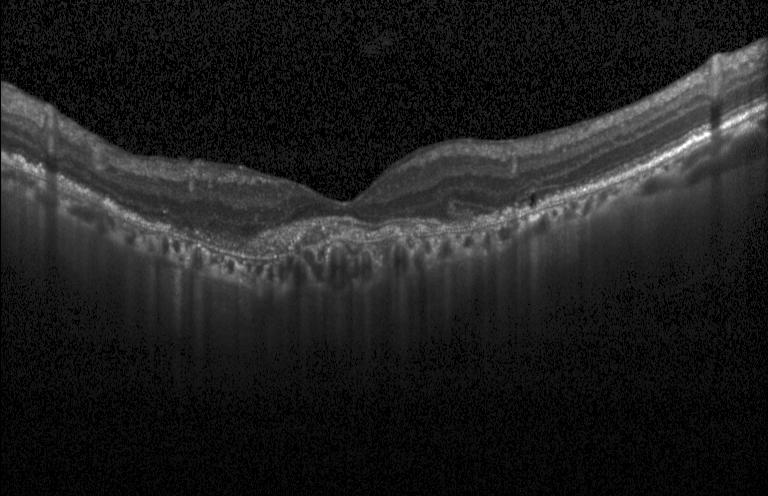

Optical coherence tomography scan. Spectral-domain optical coherence tomography
A choroidal neovascular membrane.